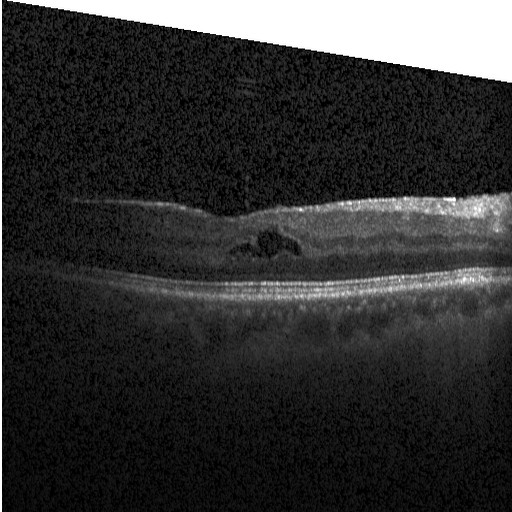 OCT finding: DME.